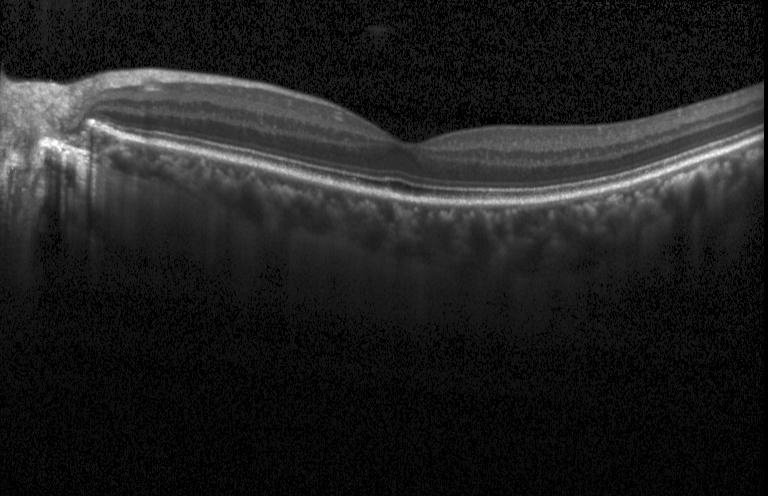 Spectral-domain OCT B-scan: neither choroidal neovascularization, diabetic macular edema, nor drusen.